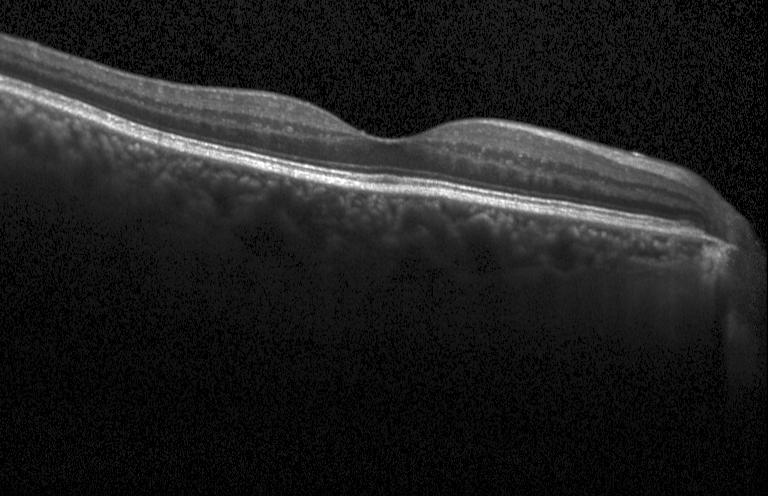

Impression: neither choroidal neovascularization, diabetic macular edema, nor drusen.